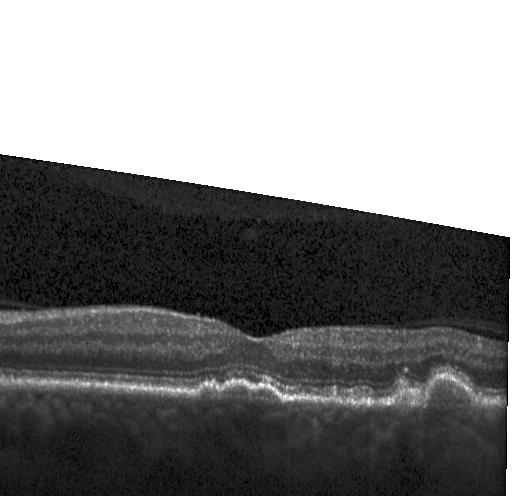

Spectral-domain OCT; OCT B-scan
This B-scan demonstrates sub-RPE drusenoid deposits.